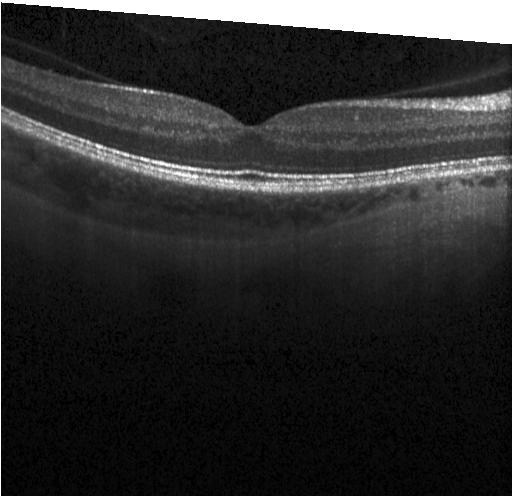
Heidelberg Spectralis OCT system · macular scan · retinal OCT B-scan
No choroidal neovascularization, no diabetic macular edema, and no drusen.